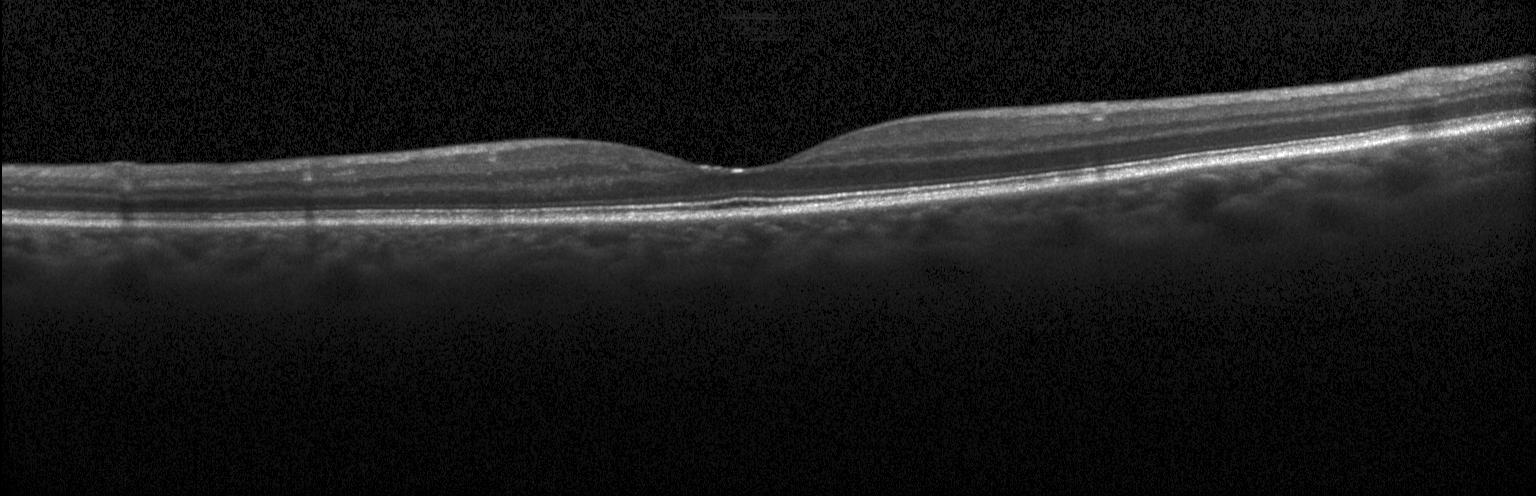

Horizontal scan through the fovea; instrument: Heidelberg Spectralis; retinal OCT B-scan; SD-OCT. Neither CNV, DME, nor drusen.